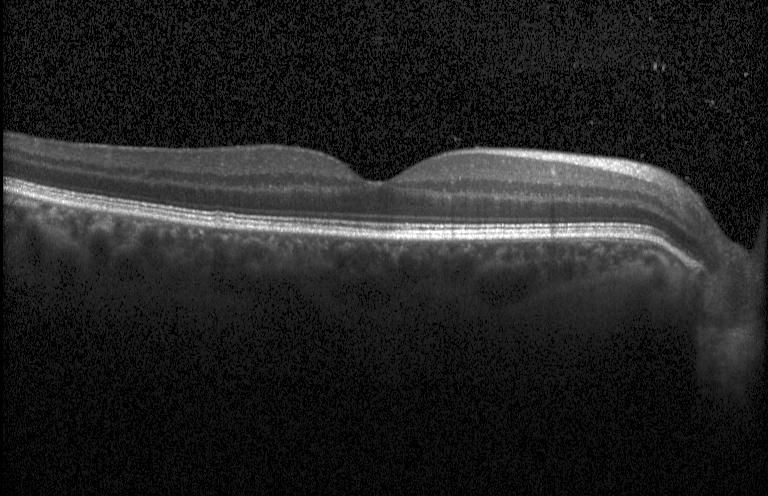
Spectral-domain optical coherence tomography, OCT line scan — Diagnosis: neither CNV, DME, nor drusen.